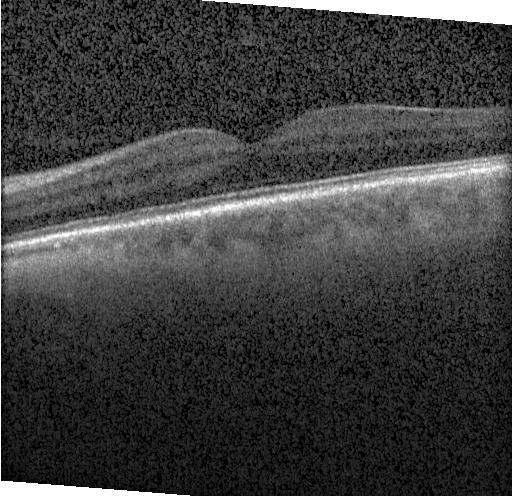 Optical coherence tomography scan, centered on the fovea, acquired on a Heidelberg Spectralis, spectral-domain optical coherence tomography
Diagnosis: no CNV, DME, or drusen.